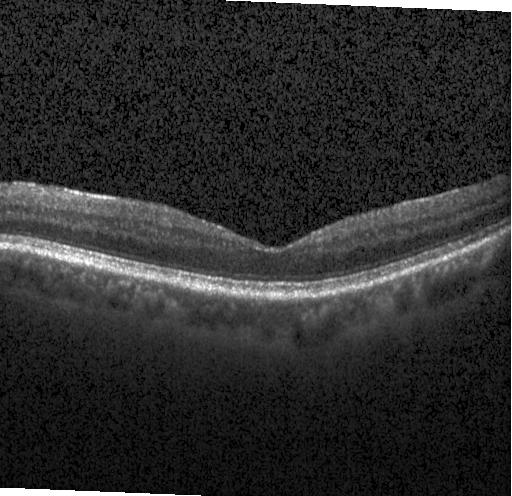

Retinal OCT cross-section.
Impression: no choroidal neovascularization, diabetic macular edema, or drusen.